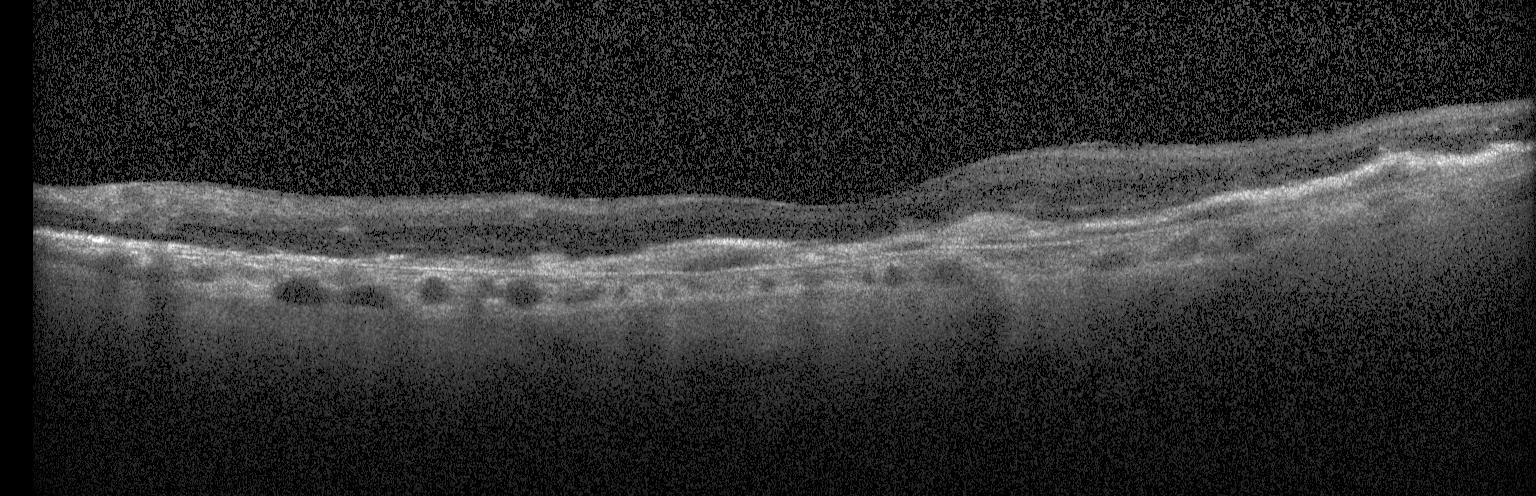 Retinal OCT cross-section
Diagnosis: a choroidal neovascular membrane.